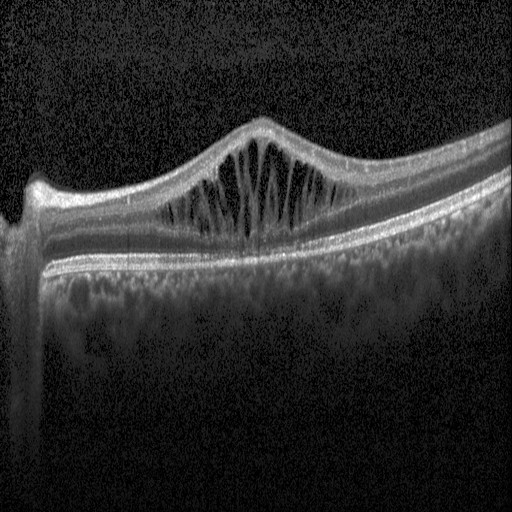 Retinal OCT cross-section — The scan shows diabetic macular edema.